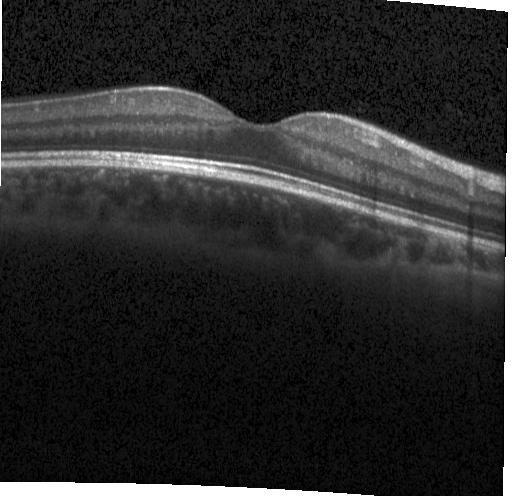 Spectral-domain OCT B-scan: no CNV, no DME, and no drusen.